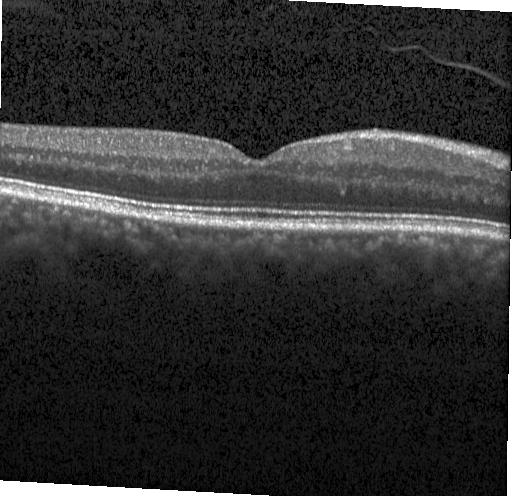
Spectral-domain OCT, acquired on a Heidelberg Spectralis, optical coherence tomography scan. Impression: no choroidal neovascularization, no diabetic macular edema, and no drusen.